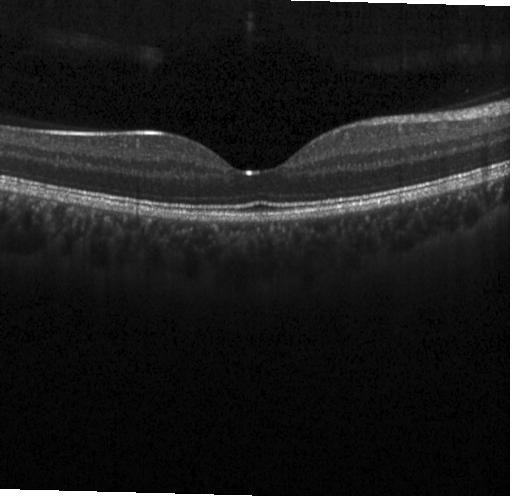
Acquired on a Heidelberg Spectralis · OCT line scan
Impression: no choroidal neovascularization, no diabetic macular edema, and no drusen.